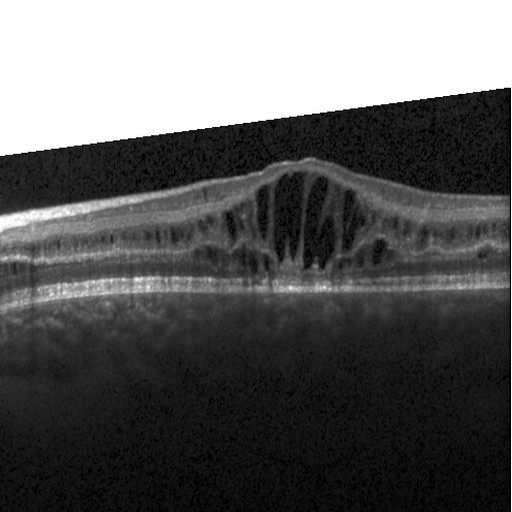
Spectral-domain optical coherence tomography, retinal OCT cross-section.
This B-scan demonstrates diabetic macular edema (DME).